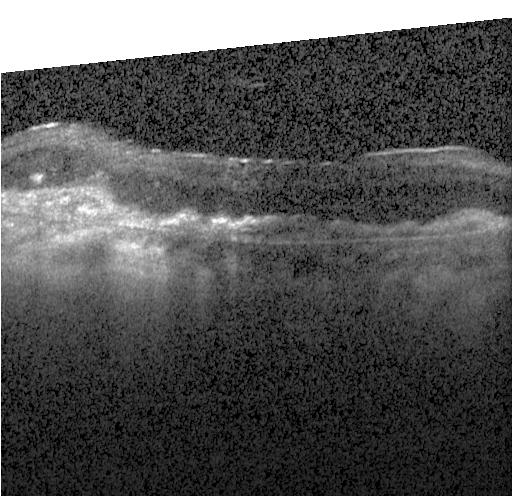
Dx: a choroidal neovascular membrane.